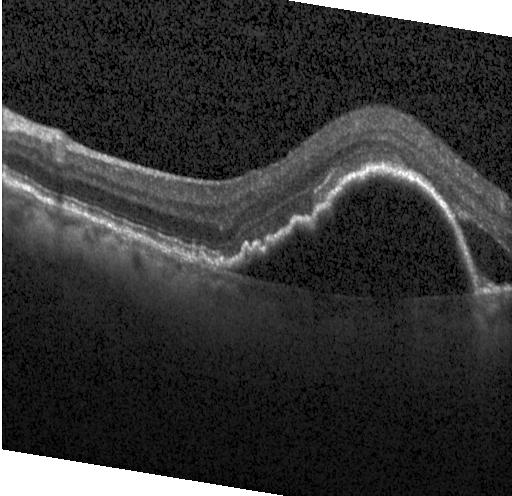
OCT scan showing CNV.